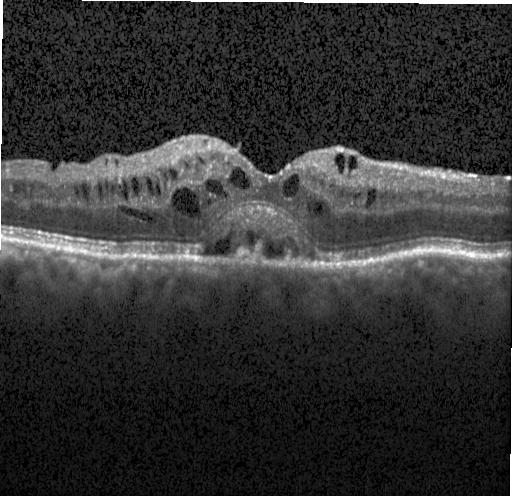 Acquired on a Heidelberg Spectralis; OCT line scan. Macular OCT: diabetic macular edema.